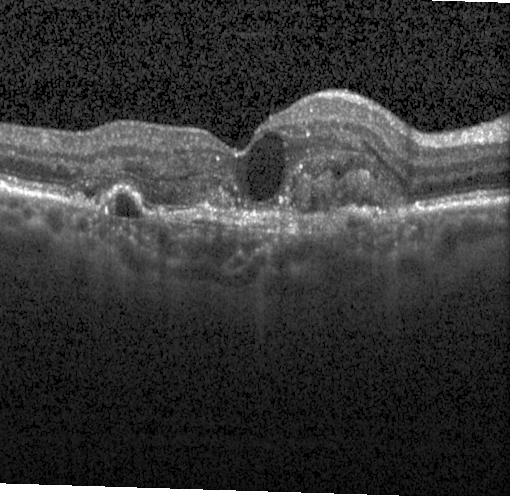 Spectral-domain OCT · optical coherence tomography scan · macular scan · acquired on a Heidelberg Spectralis — OCT finding: choroidal neovascularization (CNV).